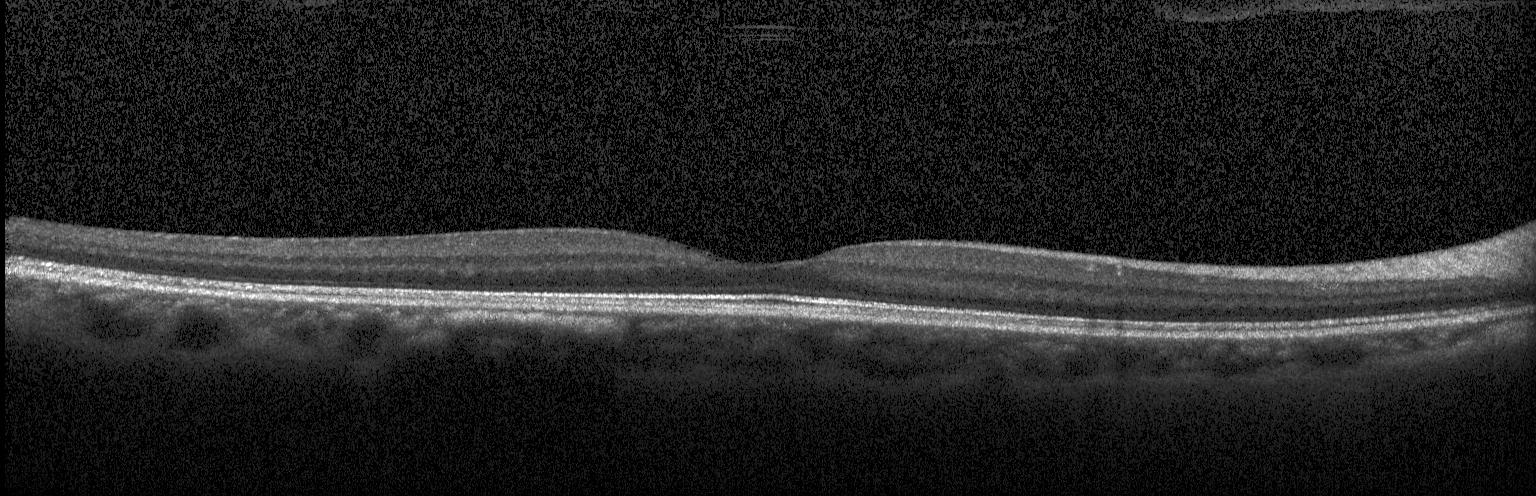 Spectral-domain OCT, Heidelberg Spectralis OCT system, optical coherence tomography scan
Dx: no evidence of CNV, DME, or drusen.